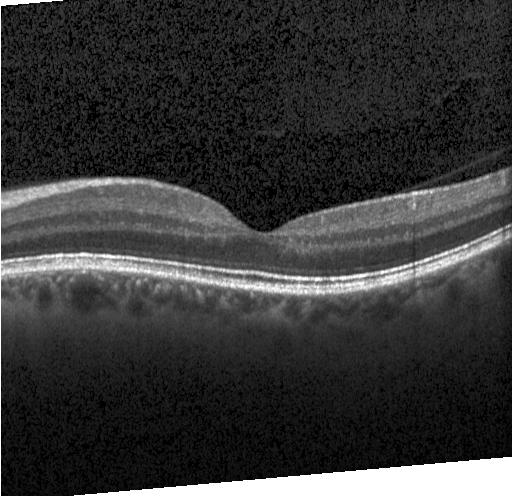
Retinal OCT B-scan.
Diagnosis: no CNV, no DME, and no drusen.